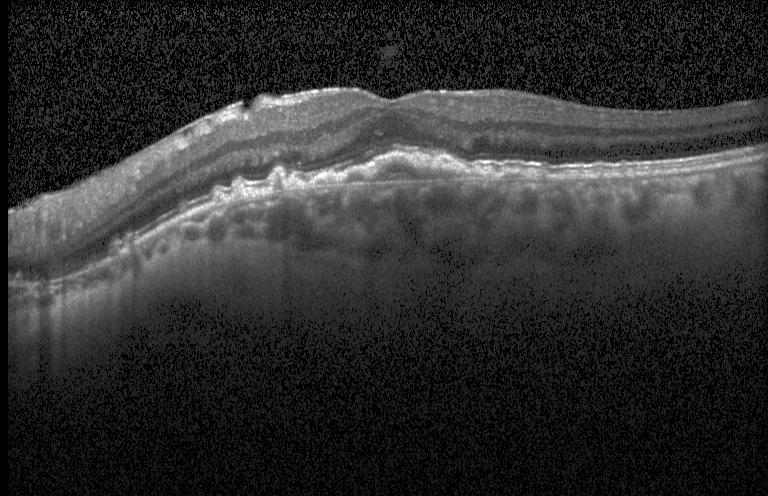

Instrument: Heidelberg Spectralis. Retinal OCT cross-section. Macular scan
Diagnosis: choroidal neovascularization (CNV).